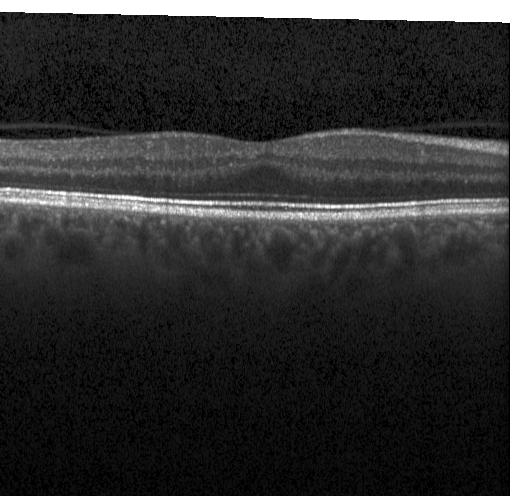

Macular OCT: no CNV, DME, or drusen.